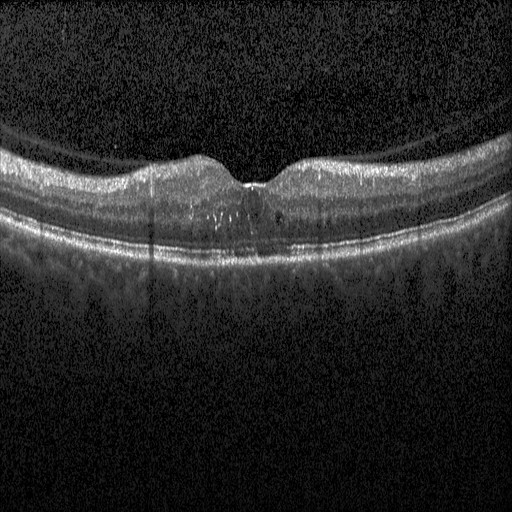 SD-OCT; OCT B-scan; horizontal scan through the fovea. Impression: diabetic macular edema (DME).